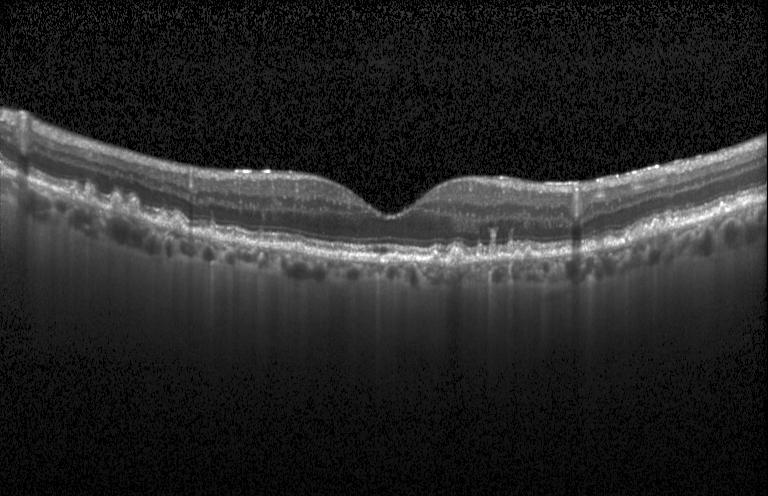 Macular OCT demonstrating multiple drusen.